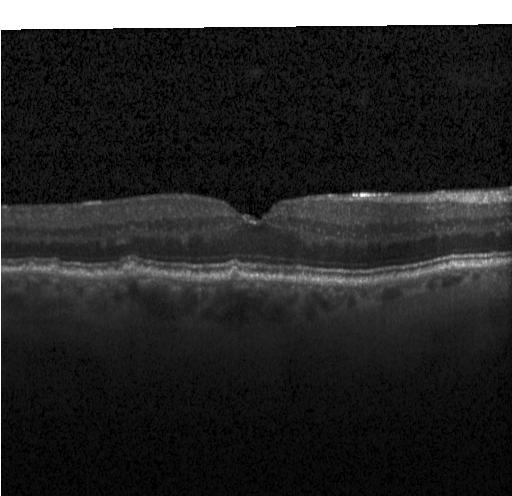 Acquired on a Heidelberg Spectralis; horizontal scan through the fovea; OCT B-scan. Assessment: multiple drusen.